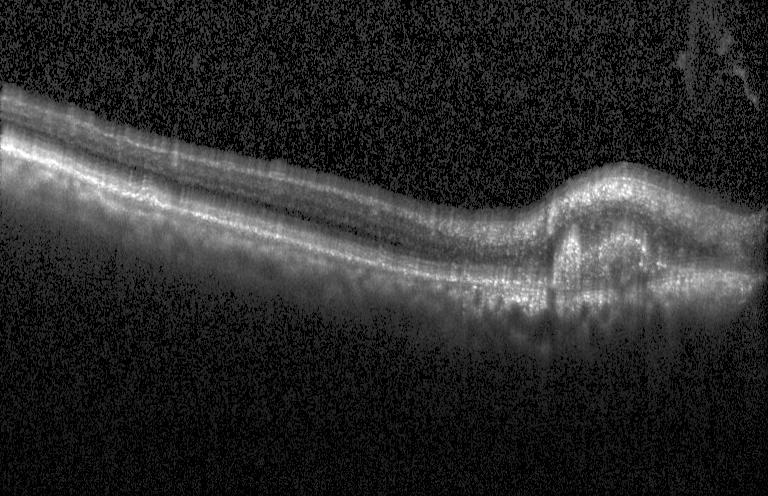 Retinal OCT cross-section
Impression: choroidal neovascularization (CNV).